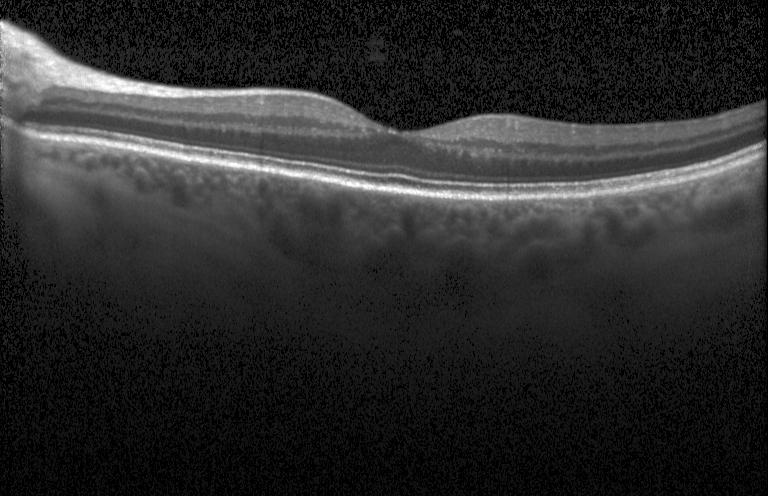
Acquired on a Heidelberg Spectralis · spectral-domain OCT · fovea-centered · optical coherence tomography B-scan.
Finding: neither choroidal neovascularization, diabetic macular edema, nor drusen.